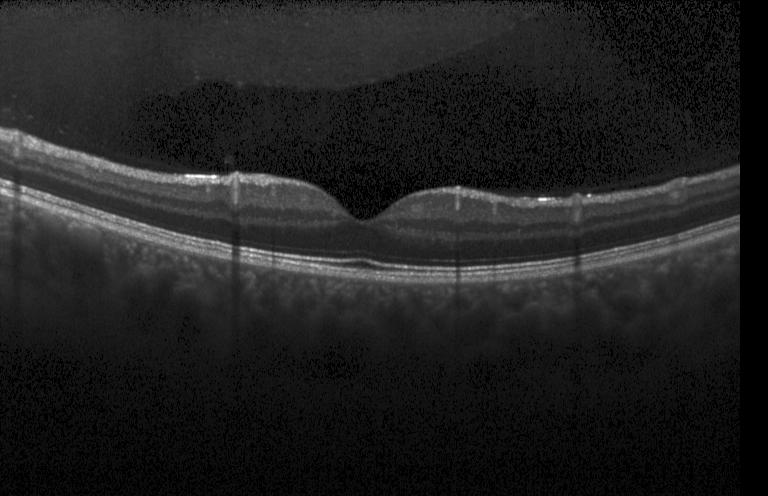

This B-scan demonstrates no evidence of choroidal neovascularization, diabetic macular edema, or drusen.